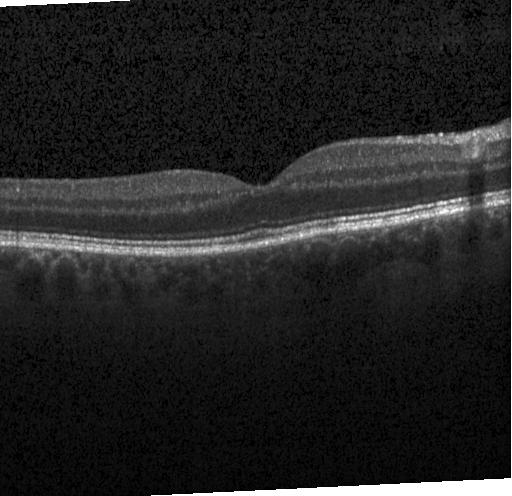 No choroidal neovascularization, diabetic macular edema, or drusen.